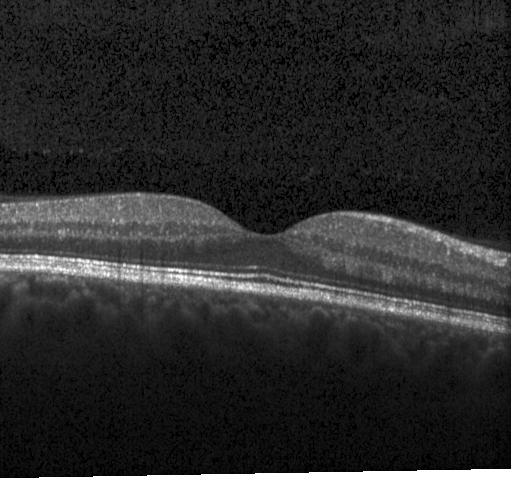
OCT B-scan — Finding: no CNV, no DME, and no drusen.